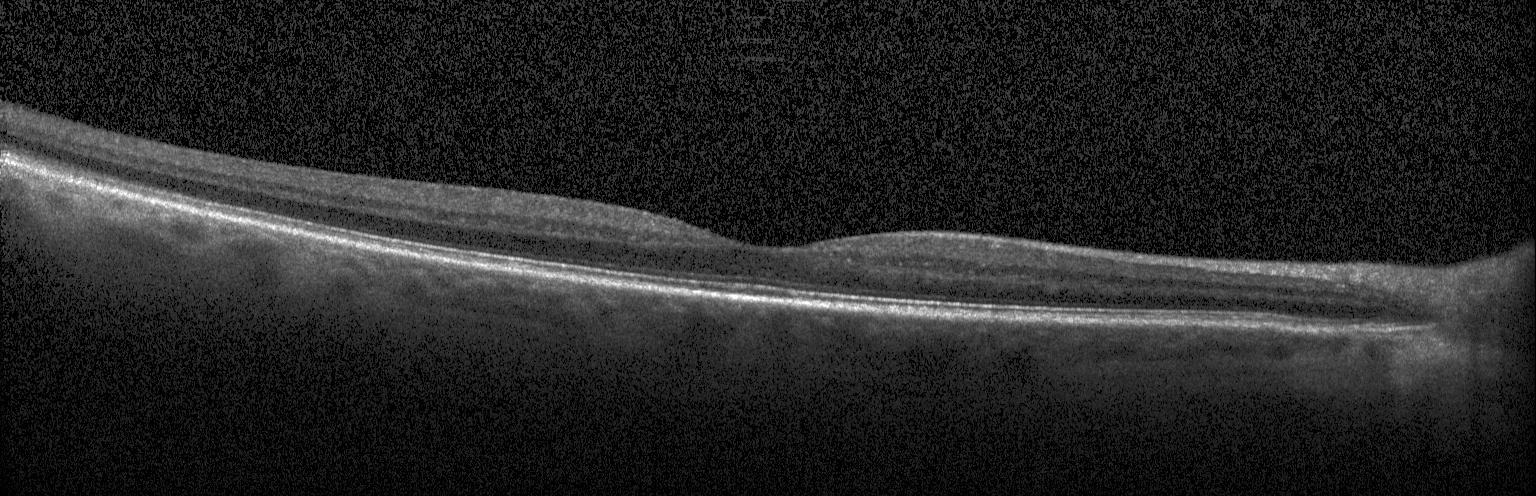
Heidelberg Spectralis OCT system; spectral-domain optical coherence tomography; horizontal scan through the fovea; optical coherence tomography B-scan — Dx: neither CNV, DME, nor drusen.